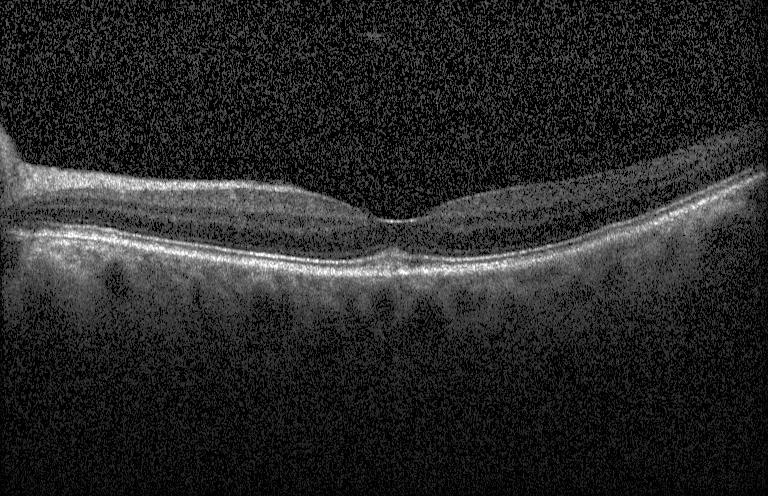
Macular OCT demonstrating neither choroidal neovascularization, diabetic macular edema, nor drusen.